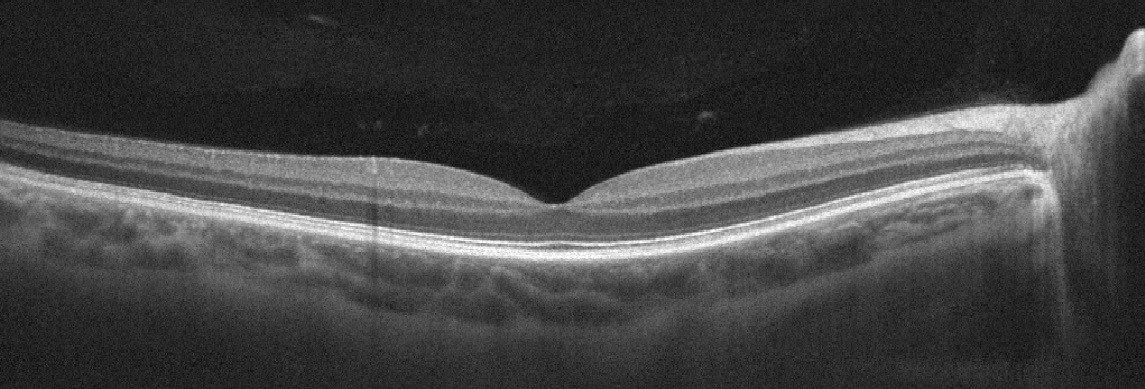 Optical coherence tomography scan, macular scan
This B-scan demonstrates absence of AMD, DME, ERM, RAO, RVO, and vitreomacular interface disease.